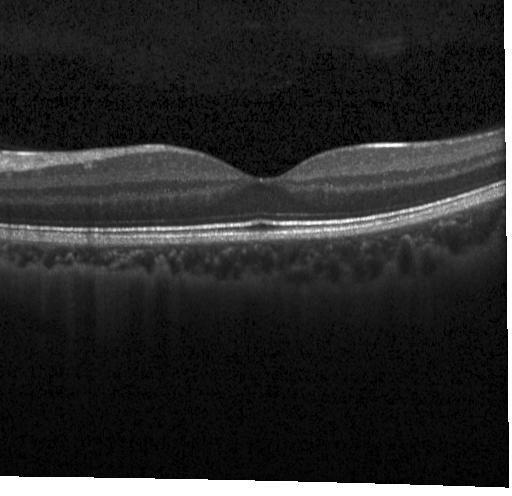

Spectral-domain optical coherence tomography. Instrument: Heidelberg Spectralis. Retinal OCT cross-section. Fovea-centered.
Diagnosis: neither CNV, DME, nor drusen.